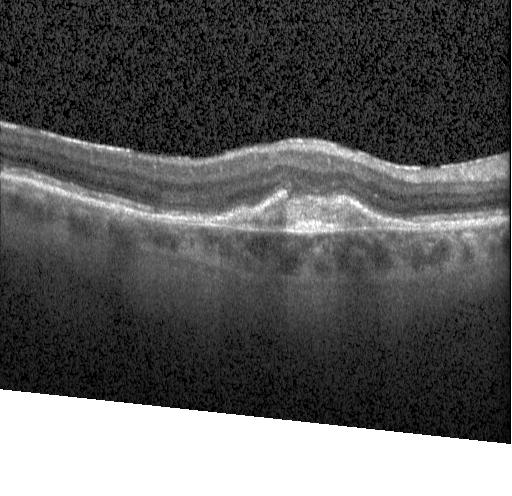

Finding: CNV.